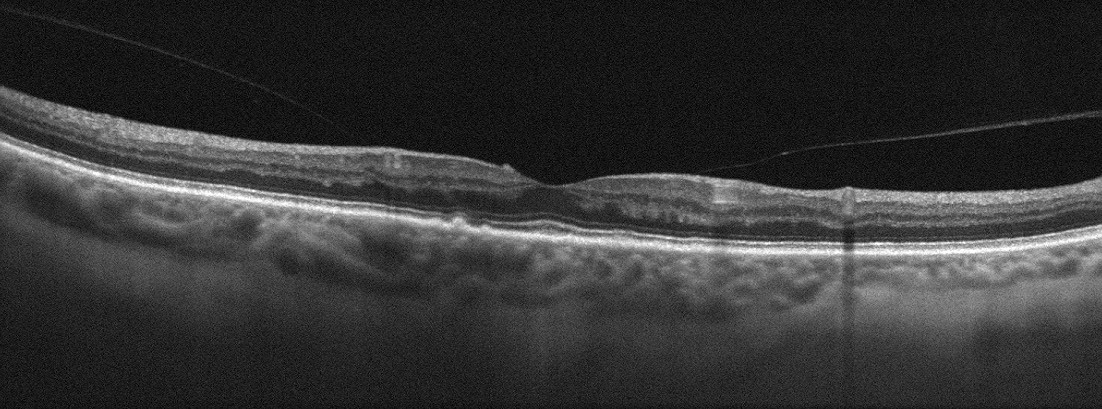
Spectral-domain OCT B-scan: age-related macular degeneration.